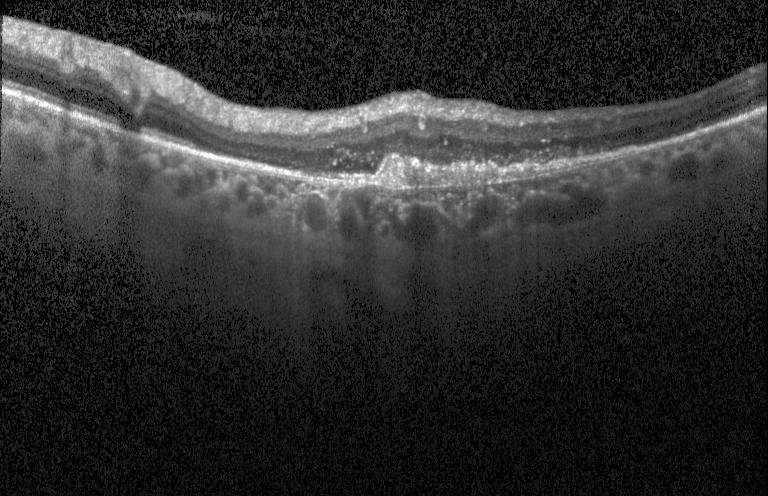 Spectral-domain optical coherence tomography. Retinal OCT B-scan.
Diagnosis: choroidal neovascularization.